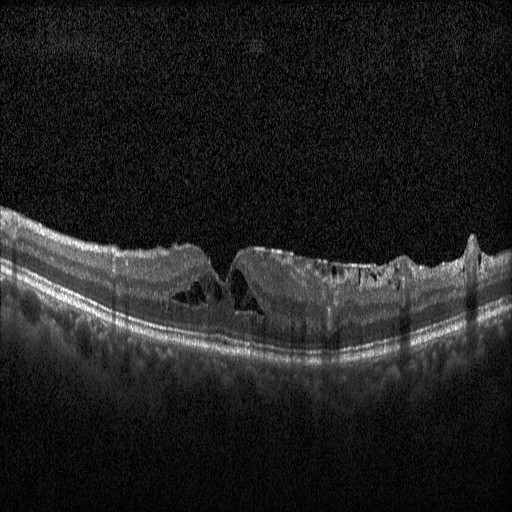 Heidelberg Spectralis, spectral-domain OCT, macular scan, optical coherence tomography scan — Finding: DME.